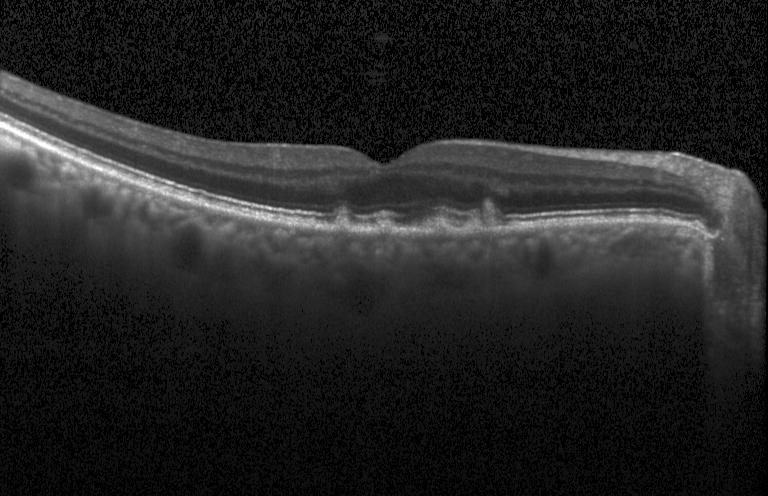
Finding: drusen.